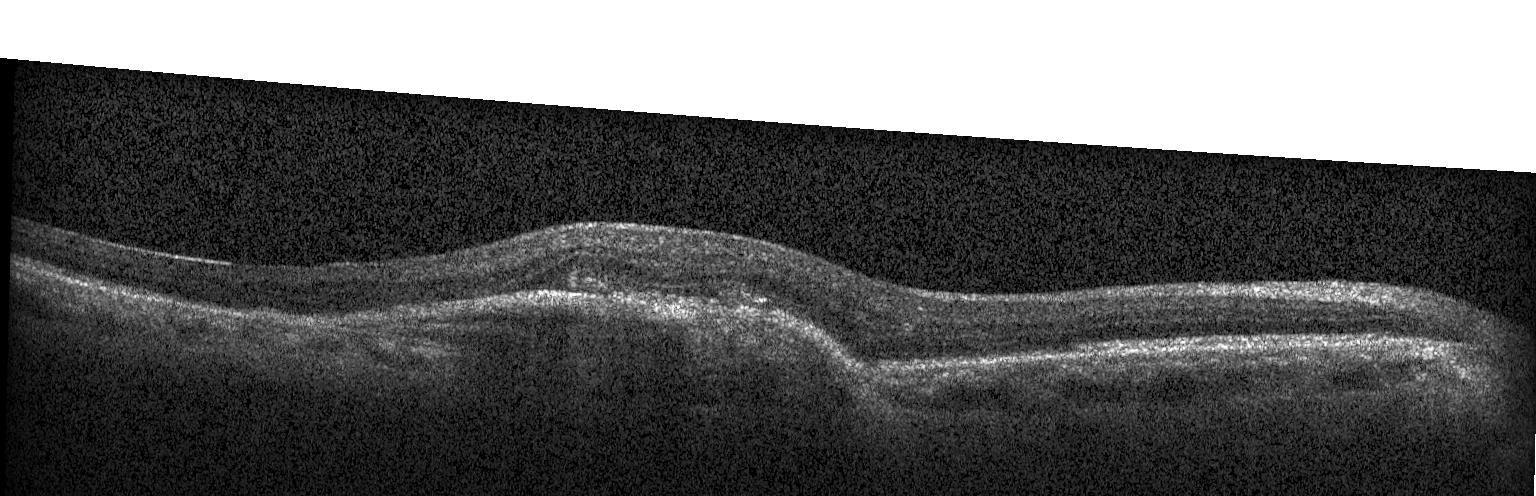

Macular scan, spectral-domain OCT, instrument: Heidelberg Spectralis, OCT line scan. Finding: a choroidal neovascular membrane.